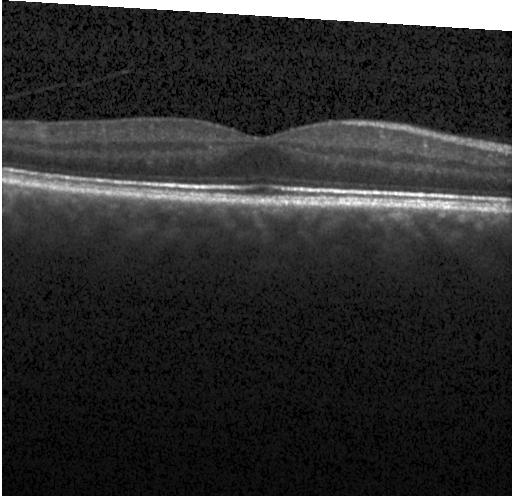

Instrument: Heidelberg Spectralis. Optical coherence tomography B-scan — Dx: no choroidal neovascularization, no diabetic macular edema, and no drusen.